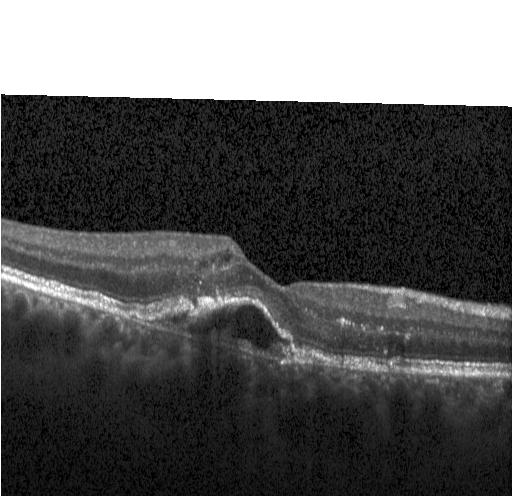

Optical coherence tomography B-scan — Finding: a choroidal neovascular membrane.